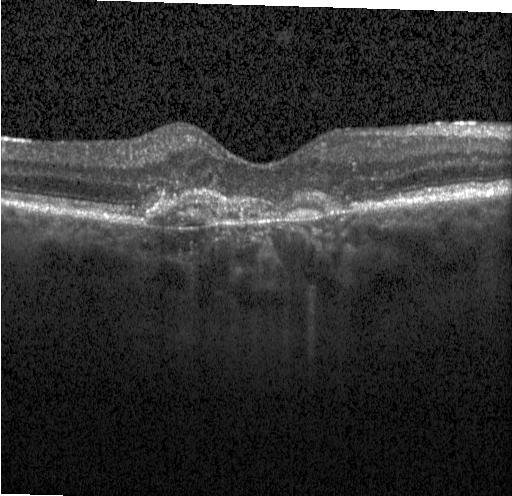

OCT scan showing choroidal neovascularization (CNV).